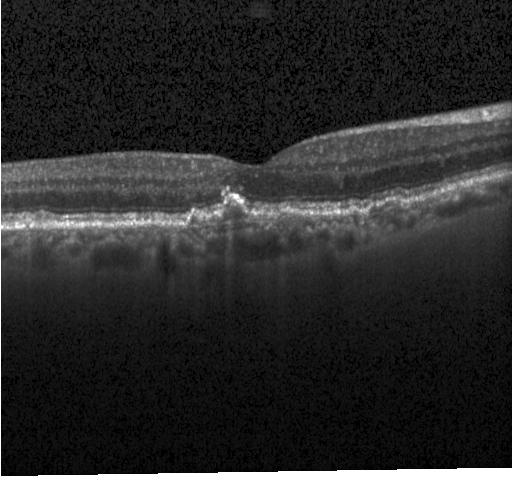
Retinal OCT cross-section showing CNV.